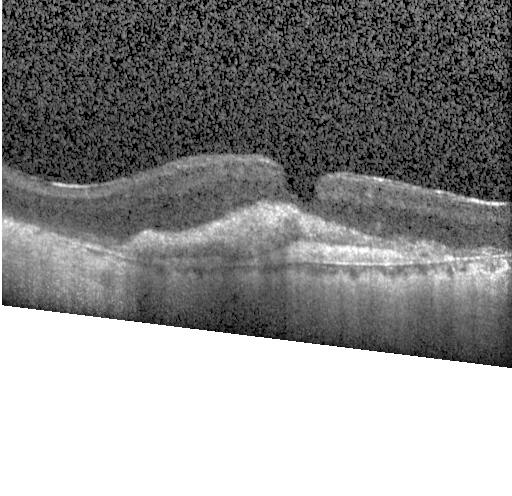 Impression: CNV.